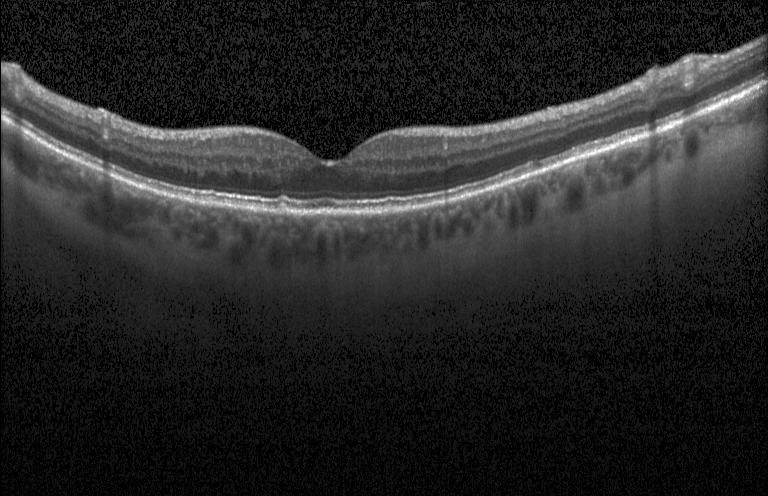 Optical coherence tomography B-scan. Heidelberg Spectralis
This B-scan demonstrates multiple drusen.